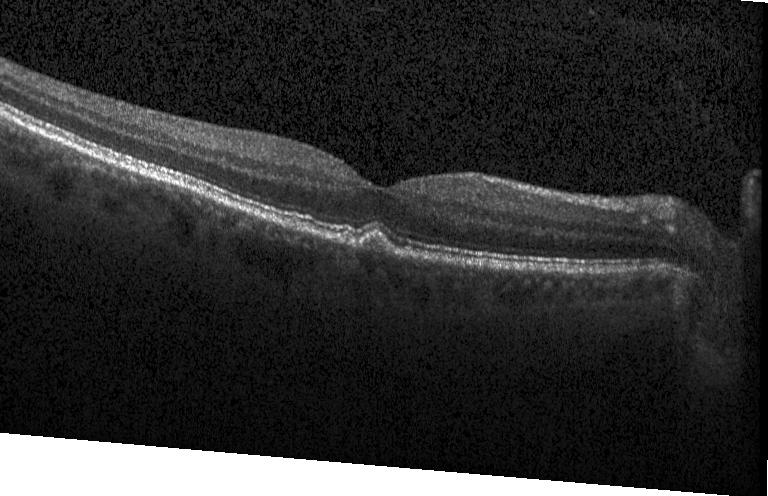 Diagnosis: sub-RPE drusenoid deposits.